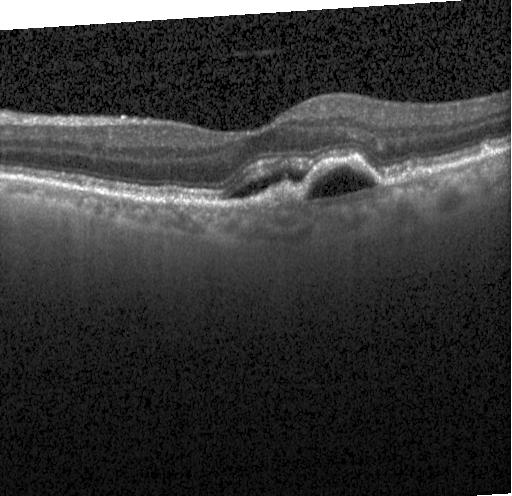

Retinal OCT B-scan
Finding: CNV.